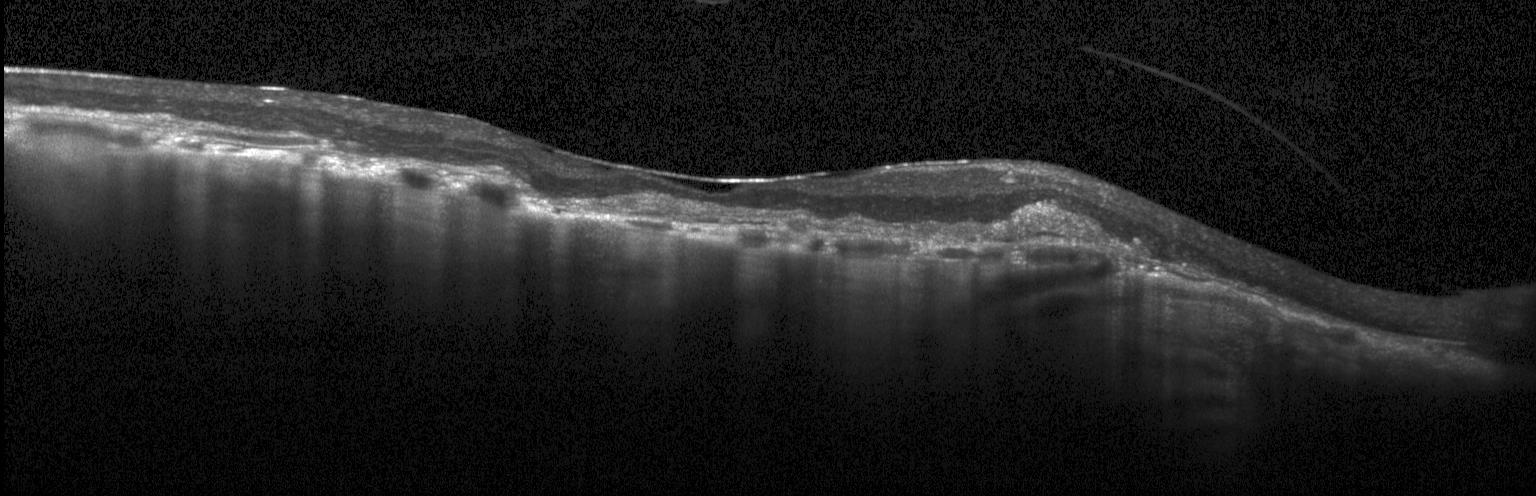

Macular OCT: choroidal neovascularization (CNV).